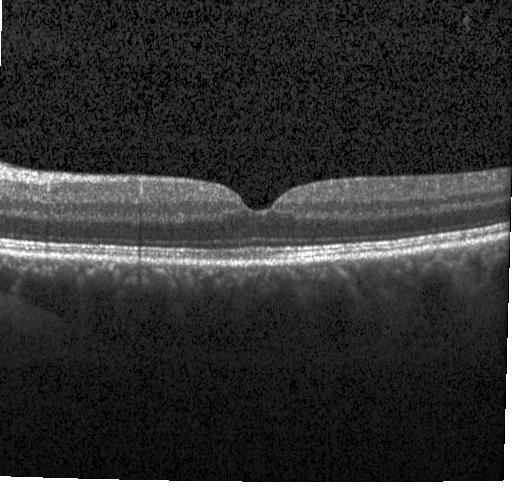
Through the macula, retinal OCT B-scan
Impression: no evidence of choroidal neovascularization, diabetic macular edema, or drusen.